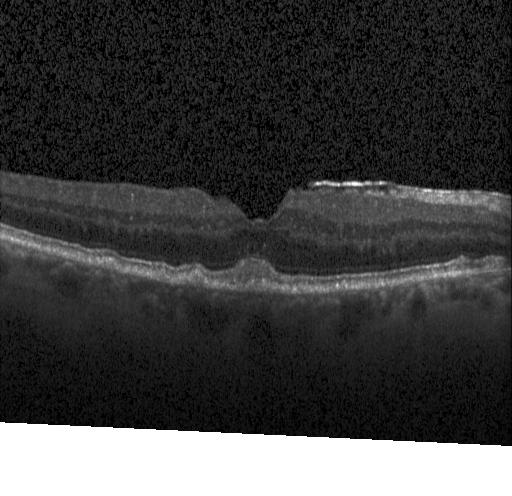
Spectral-domain OCT · optical coherence tomography B-scan · horizontal scan through the fovea
Assessment: drusen.